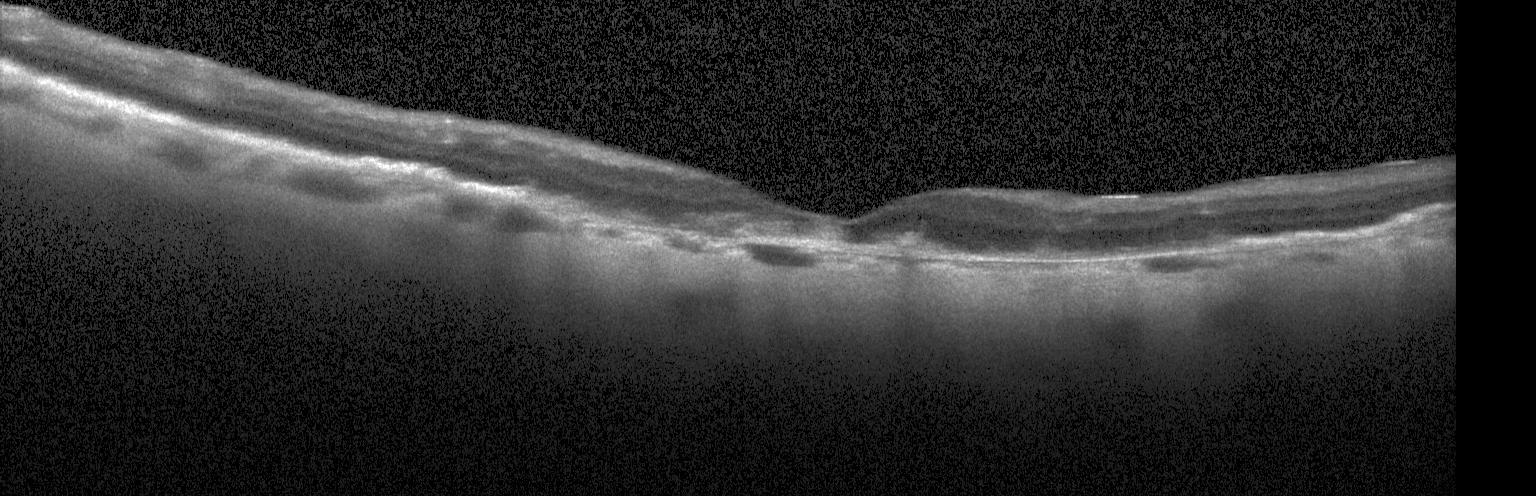 Spectral-domain OCT, optical coherence tomography scan
The scan shows choroidal neovascularization (CNV).